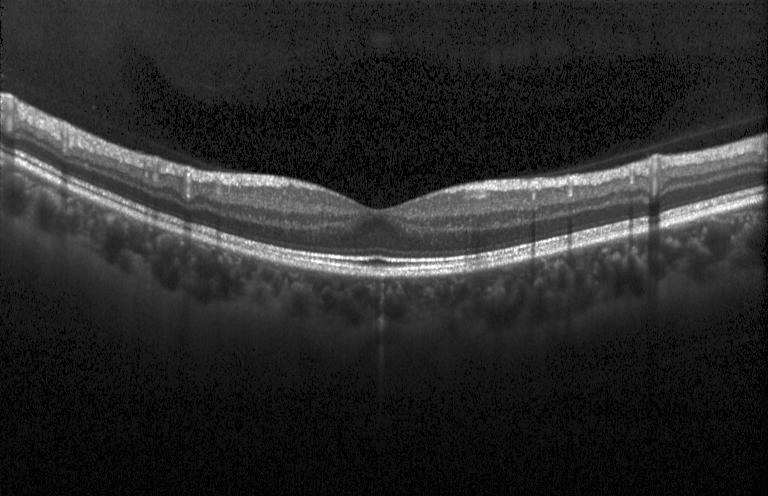

Optical coherence tomography scan · SD-OCT · acquired on a Heidelberg Spectralis · through the macula
Impression: no evidence of CNV, DME, or drusen.